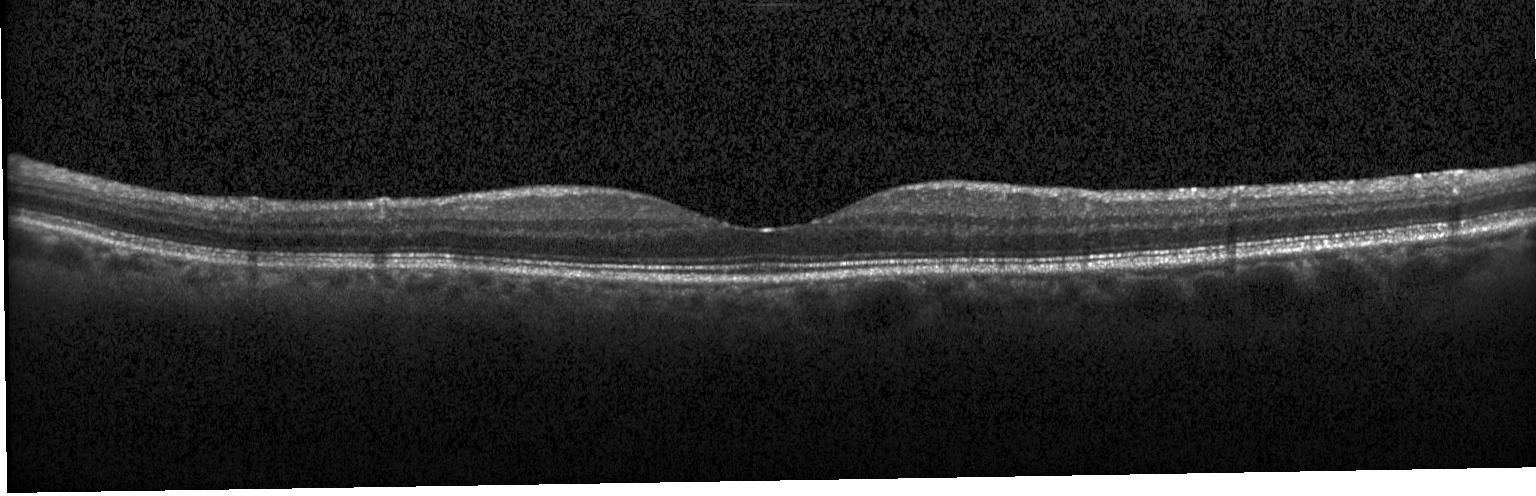 Optical coherence tomography scan — Impression: no evidence of CNV, DME, or drusen.